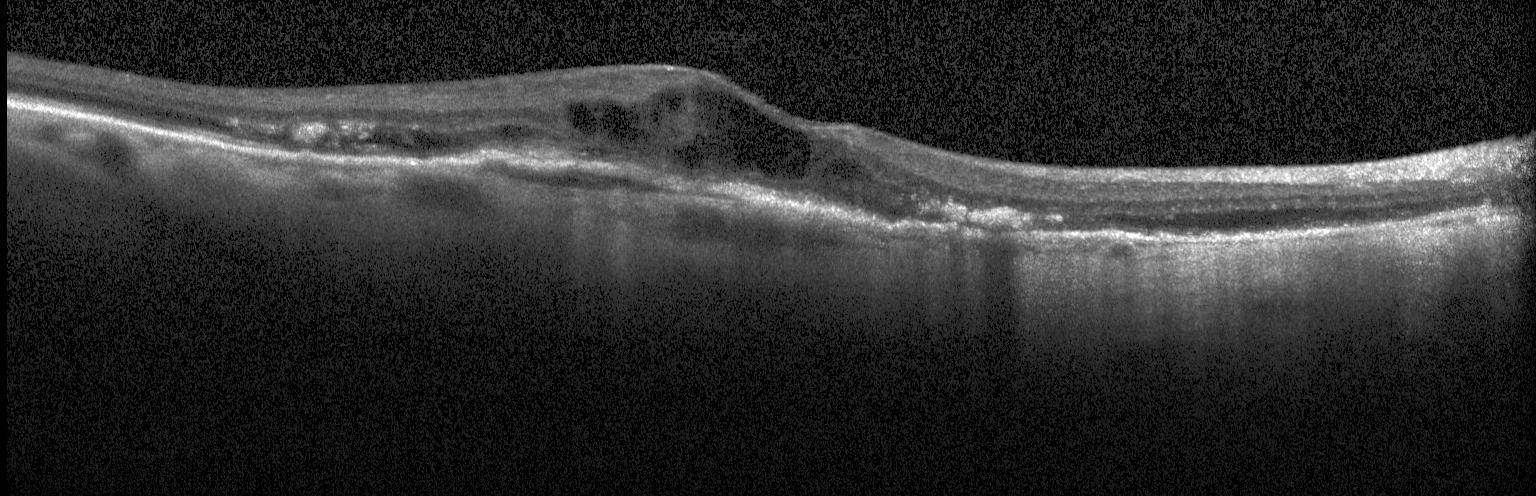 SD-OCT. Through the macula. Instrument: Heidelberg Spectralis. Retinal OCT B-scan.
Assessment: choroidal neovascularization (CNV).